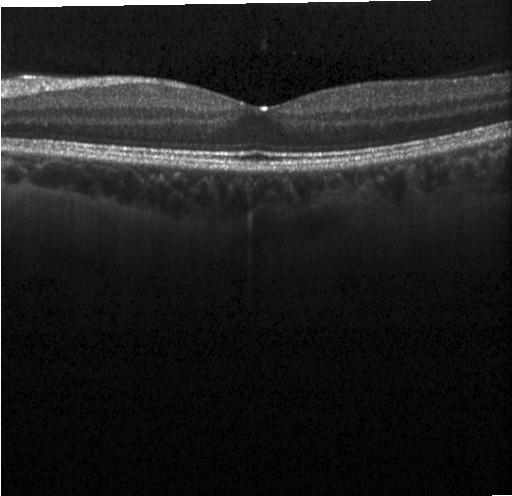 Spectral-domain OCT · OCT B-scan — Finding: neither choroidal neovascularization, diabetic macular edema, nor drusen.